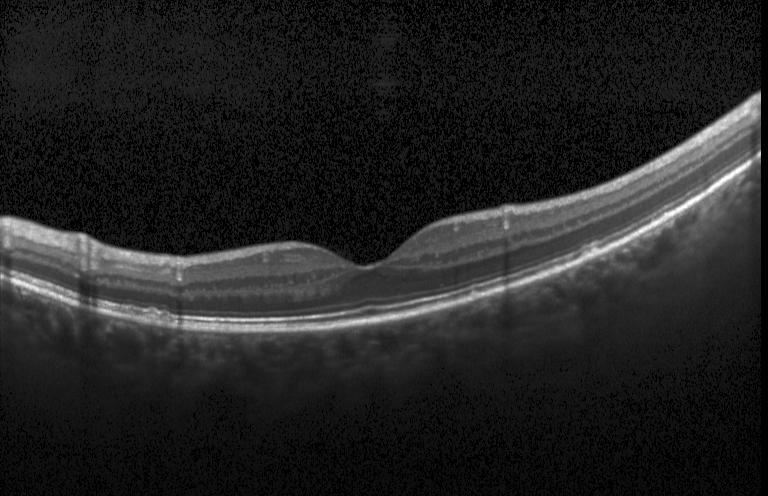
Assessment: no evidence of choroidal neovascularization, diabetic macular edema, or drusen.